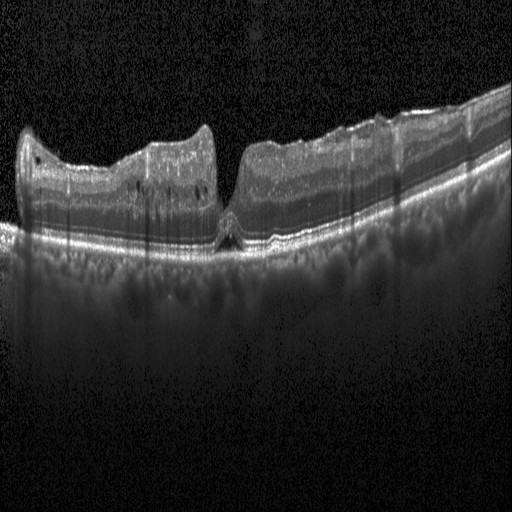
SD-OCT, Heidelberg Spectralis, retinal OCT cross-section, fovea-centered.
The scan shows diabetic macular edema.